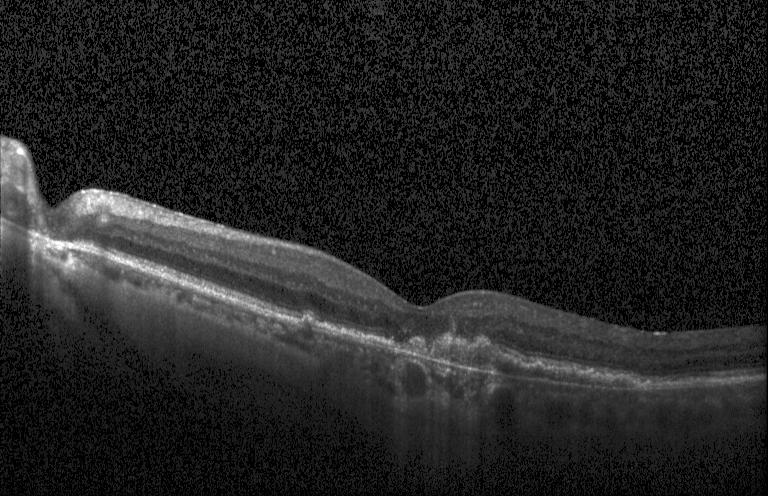

OCT finding: choroidal neovascularization.